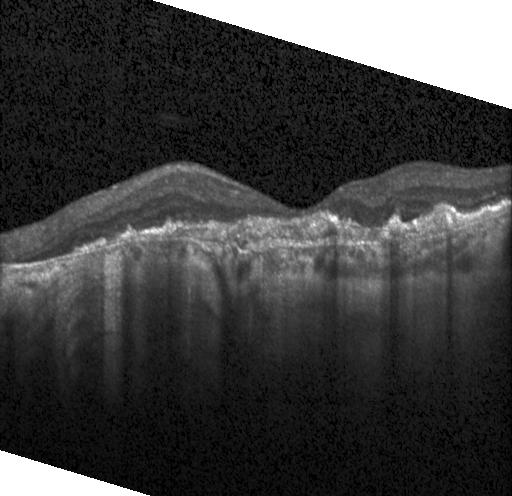

OCT finding: choroidal neovascularization.